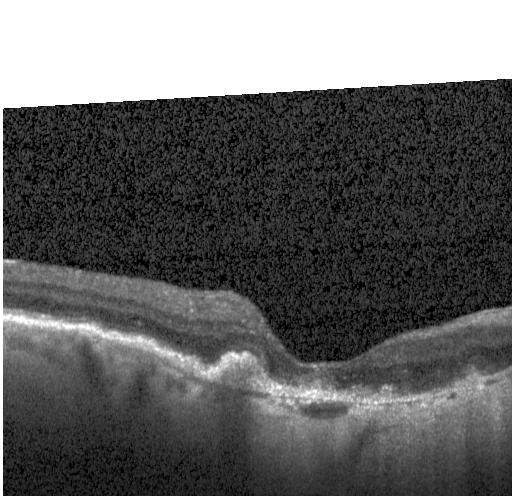 Impression: CNV.